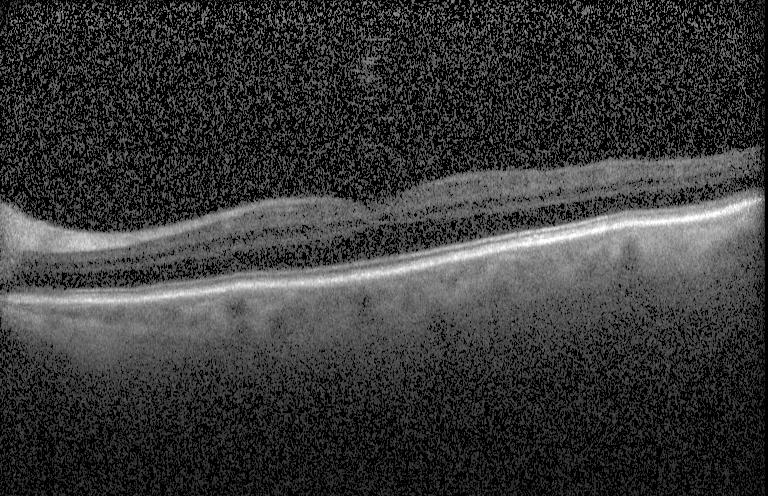

OCT line scan · spectral-domain optical coherence tomography · fovea-centered · Heidelberg Spectralis OCT system. This B-scan demonstrates no evidence of choroidal neovascularization, diabetic macular edema, or drusen.